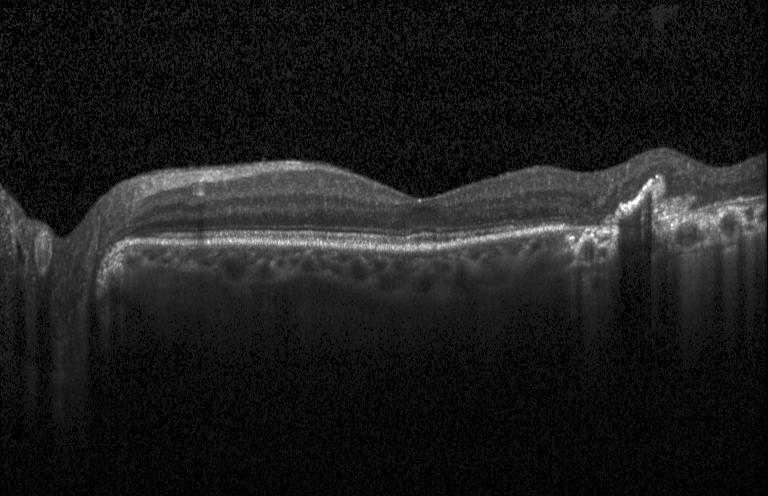

Diagnosis: a choroidal neovascular membrane.